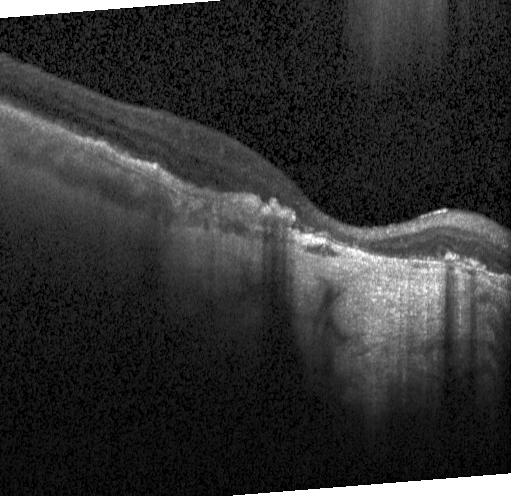 OCT B-scan.
Finding: CNV.